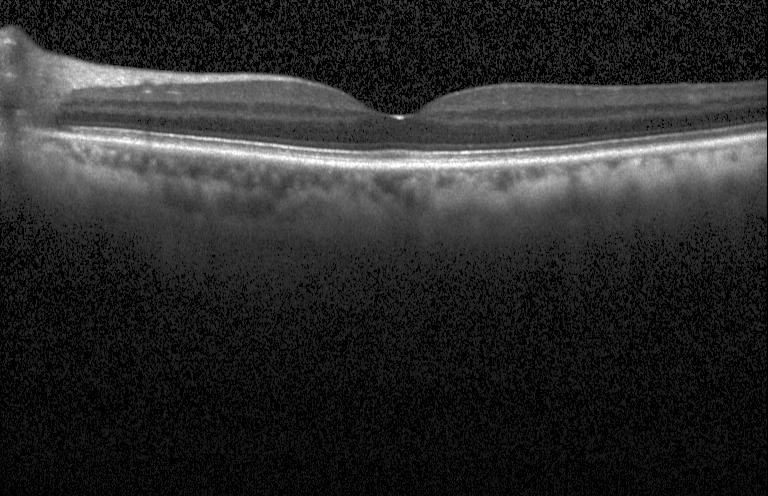 Centered on the fovea · retinal OCT B-scan · spectral-domain OCT
Diagnosis: no evidence of CNV, DME, or drusen.